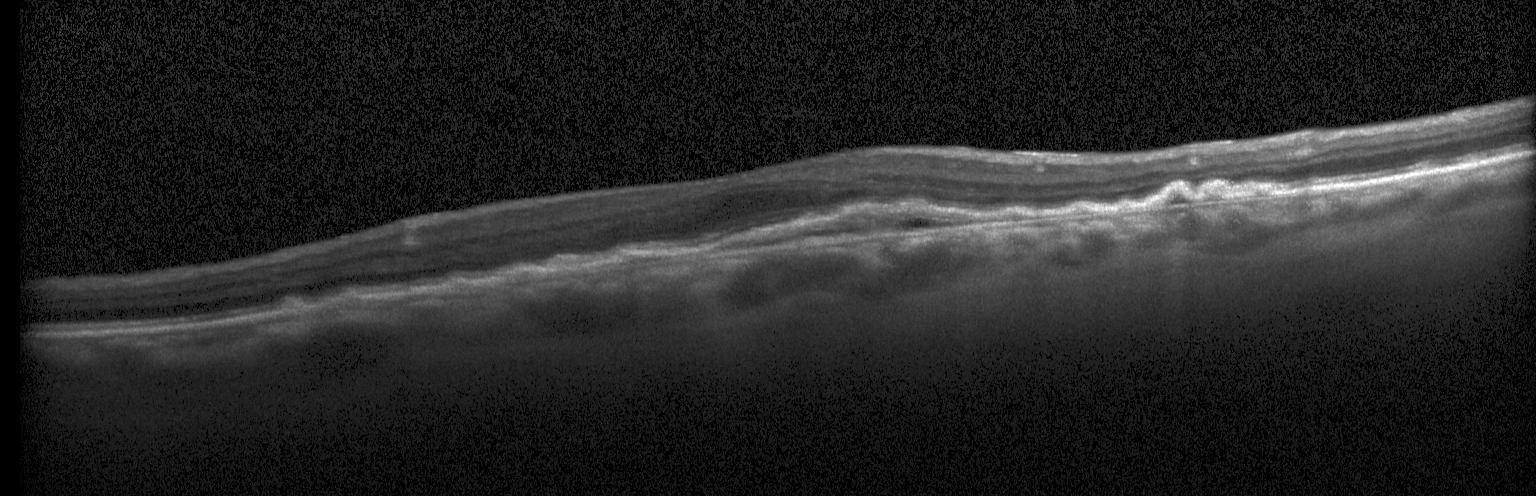

OCT scan showing CNV.